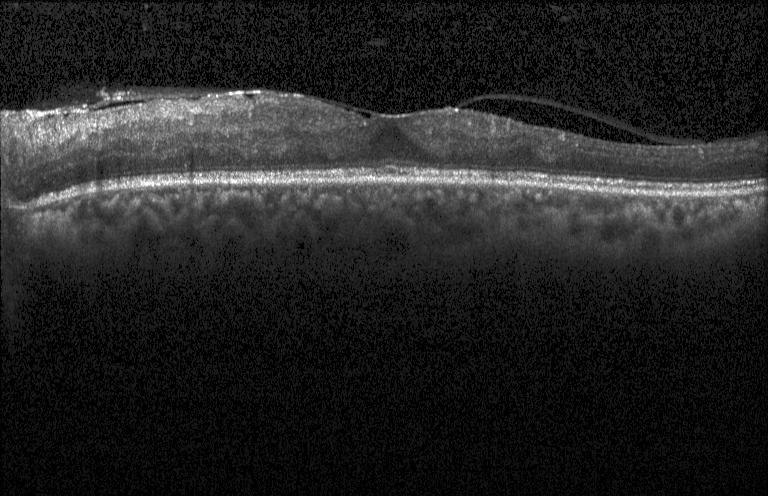 Through the macula; acquired on a Heidelberg Spectralis; spectral-domain OCT; OCT B-scan.
Macular OCT: DME.